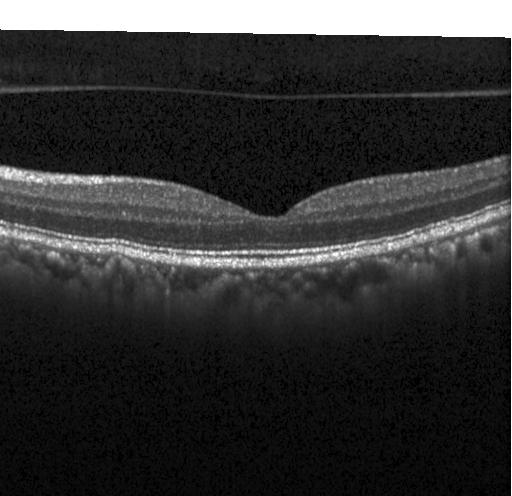

Diagnosis: no evidence of CNV, DME, or drusen.